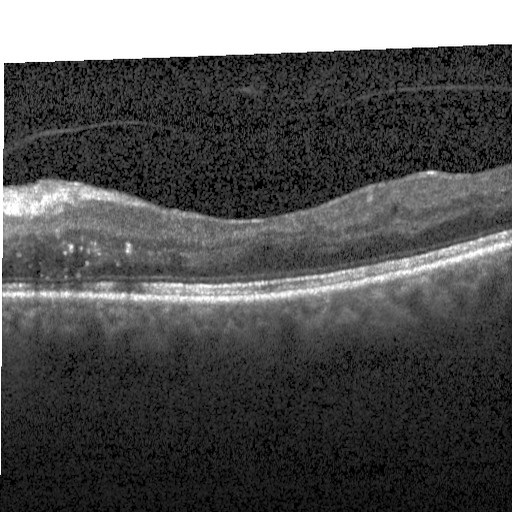 Assessment: diabetic macular edema.